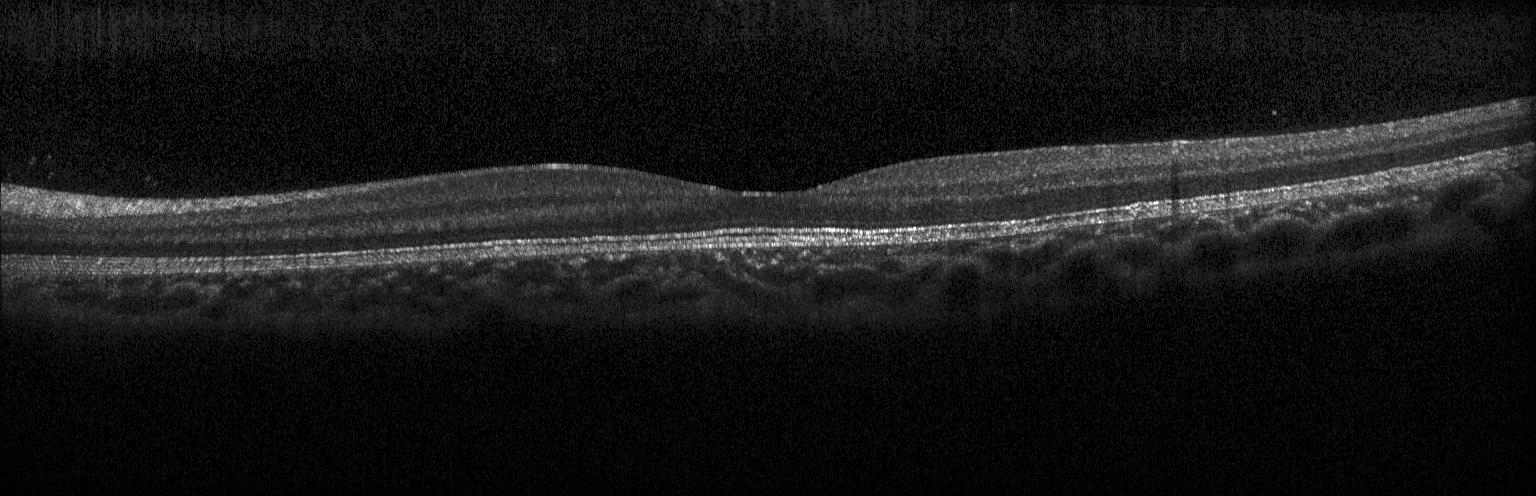

Finding: no CNV, no DME, and no drusen.